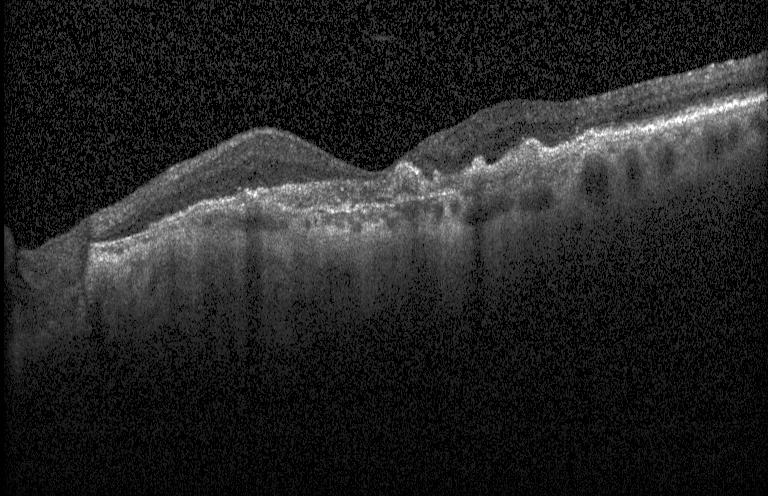

Impression: a choroidal neovascular membrane.